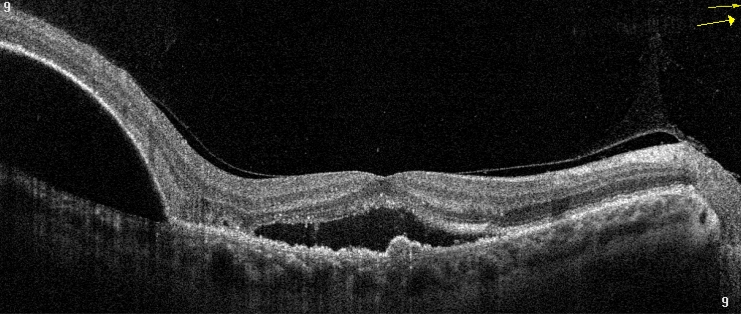
Macular scan, instrument: Optovue Avanti RTVue XR, retinal OCT B-scan — Impression: age-related macular degeneration (AMD).